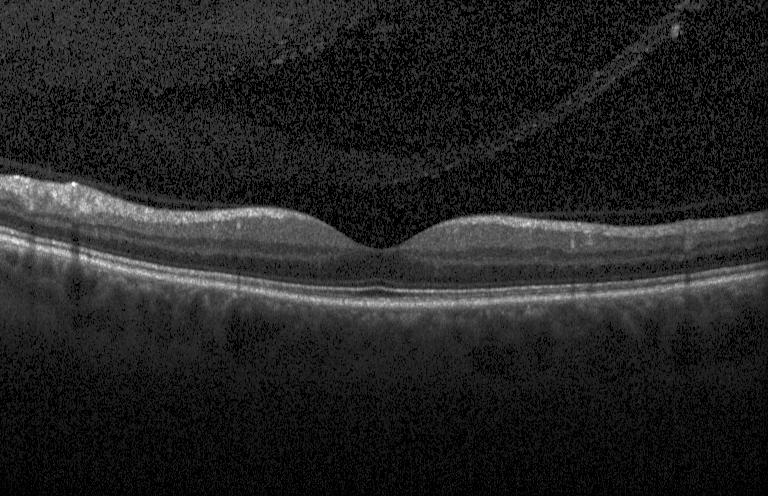

Heidelberg Spectralis OCT system, optical coherence tomography B-scan, fovea-centered, SD-OCT.
Impression: no evidence of choroidal neovascularization, diabetic macular edema, or drusen.